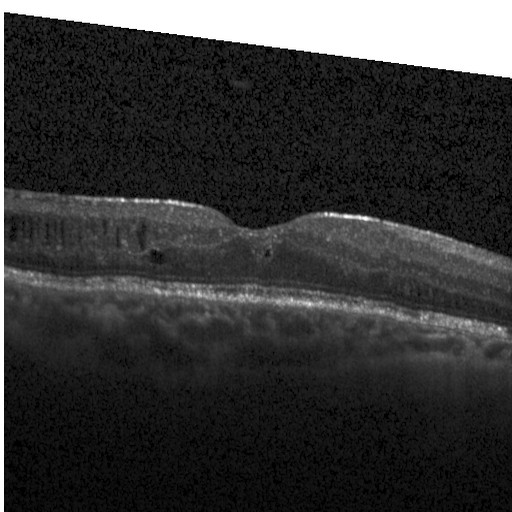

Retinal OCT B-scan · macular scan · spectral-domain optical coherence tomography.
The scan shows DME.